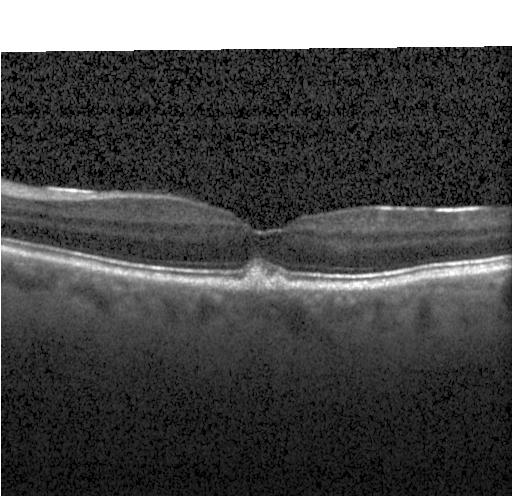 Through the macula, OCT B-scan, spectral-domain OCT, acquired on a Heidelberg Spectralis
Impression: drusen.